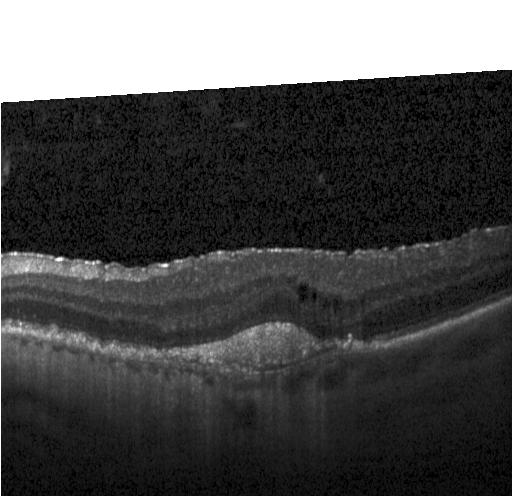 OCT line scan; spectral-domain OCT — Dx: choroidal neovascularization (CNV).